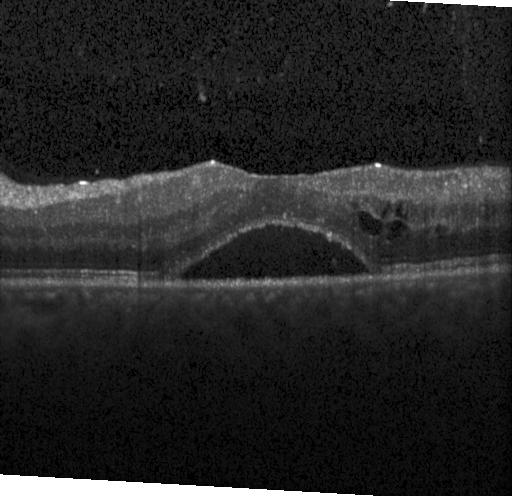

Retinal OCT B-scan; acquired on a Heidelberg Spectralis; spectral-domain optical coherence tomography; centered on the fovea — Impression: diabetic macular edema.